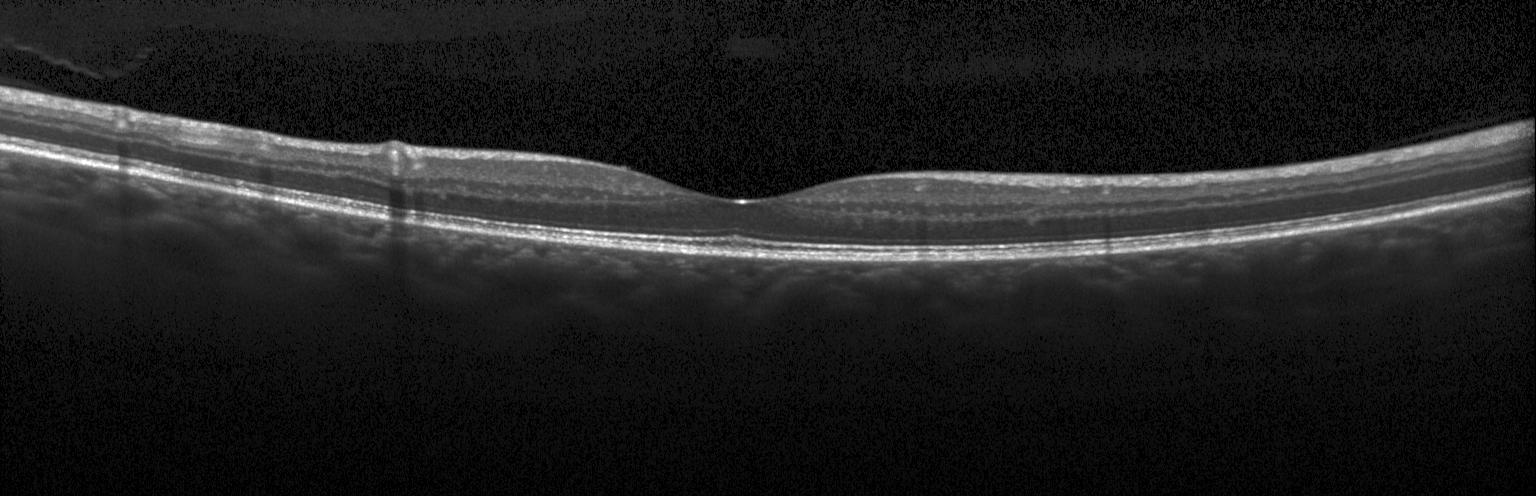 Spectral-domain OCT B-scan: no choroidal neovascularization, diabetic macular edema, or drusen.